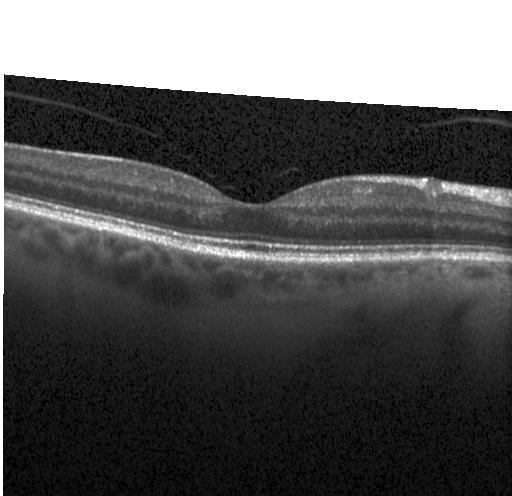
Heidelberg Spectralis OCT system; SD-OCT; retinal OCT cross-section; macular scan
The scan shows no evidence of CNV, DME, or drusen.